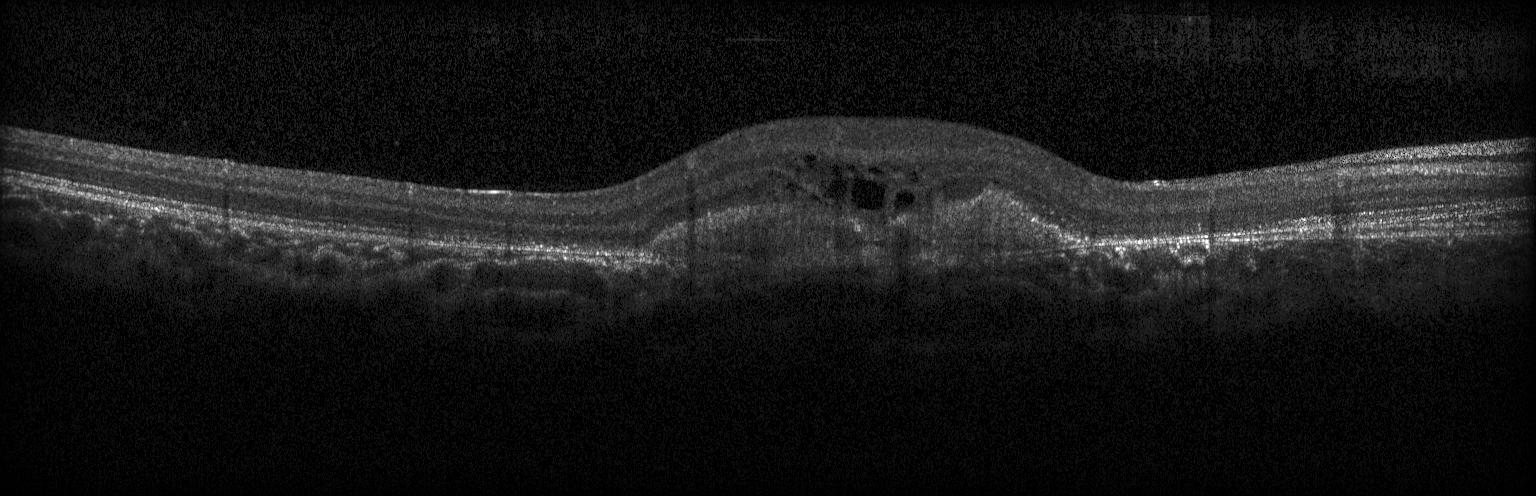

Impression: choroidal neovascularization.